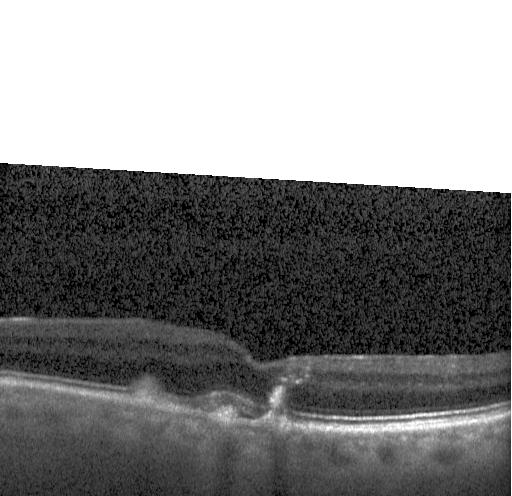
Macular OCT: choroidal neovascularization (CNV).